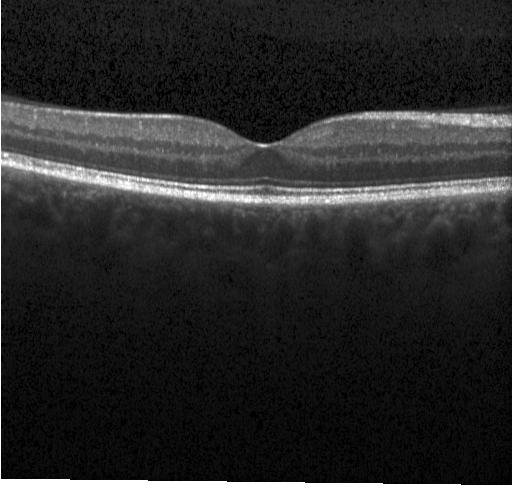
Dx: no CNV, DME, or drusen.